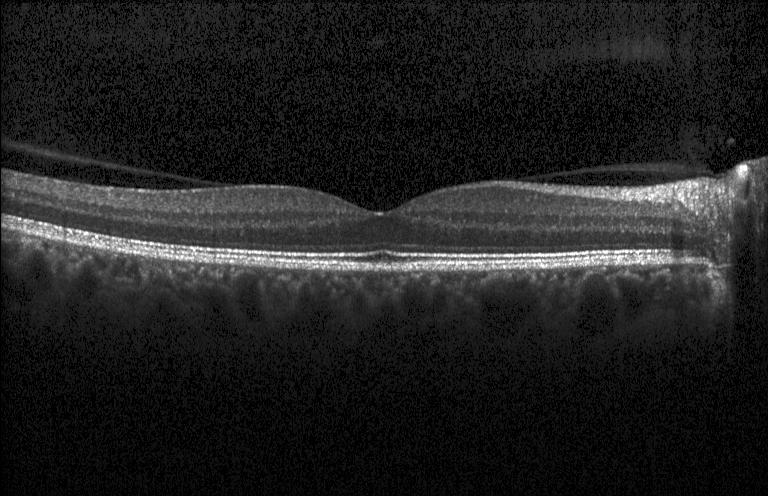
Optical coherence tomography B-scan — The scan shows neither choroidal neovascularization, diabetic macular edema, nor drusen.